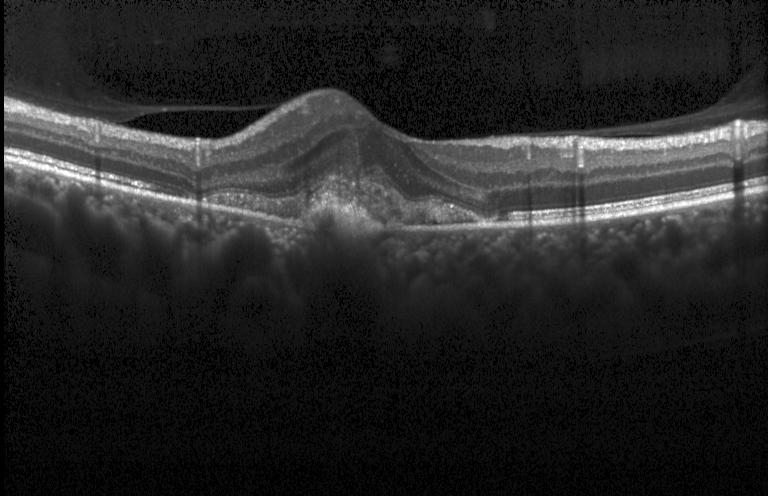 Centered on the fovea. Optical coherence tomography scan. Heidelberg Spectralis OCT system. Spectral-domain OCT
Dx: a choroidal neovascular membrane.